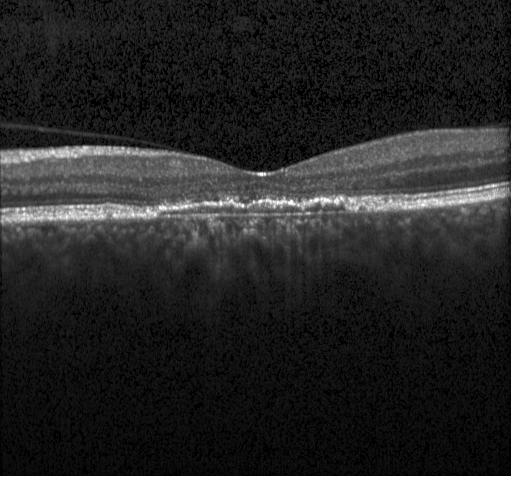
OCT B-scan, macular scan, Heidelberg Spectralis
This B-scan demonstrates a choroidal neovascular membrane.